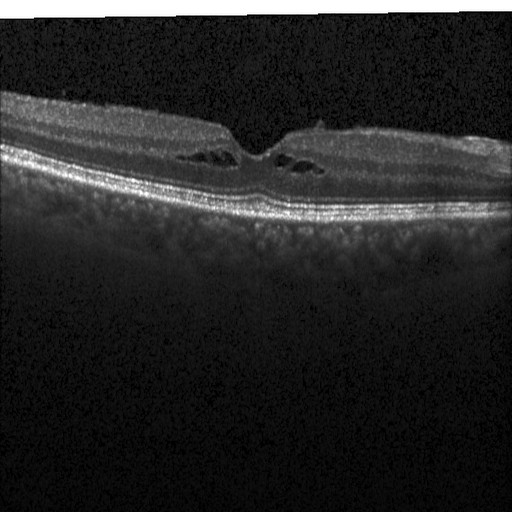
OCT line scan — Impression: diabetic macular edema (DME).